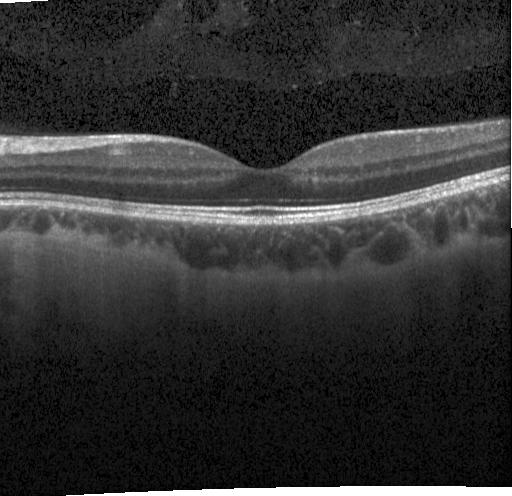

Optical coherence tomography scan; macular scan; spectral-domain optical coherence tomography; Heidelberg Spectralis — Diagnosis: no choroidal neovascularization, no diabetic macular edema, and no drusen.